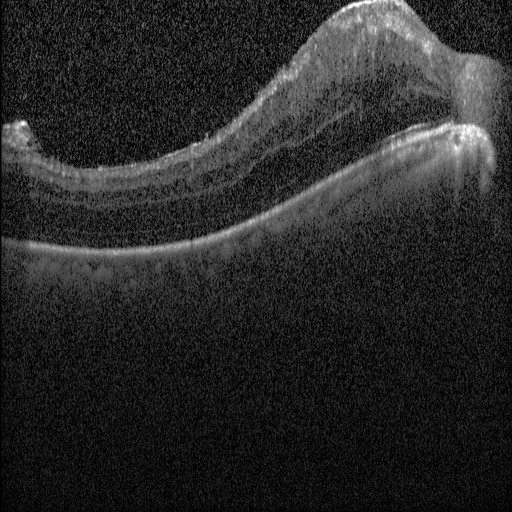
Retinal OCT cross-section; spectral-domain optical coherence tomography; Heidelberg Spectralis OCT system; fovea-centered
Dx: diabetic macular edema.